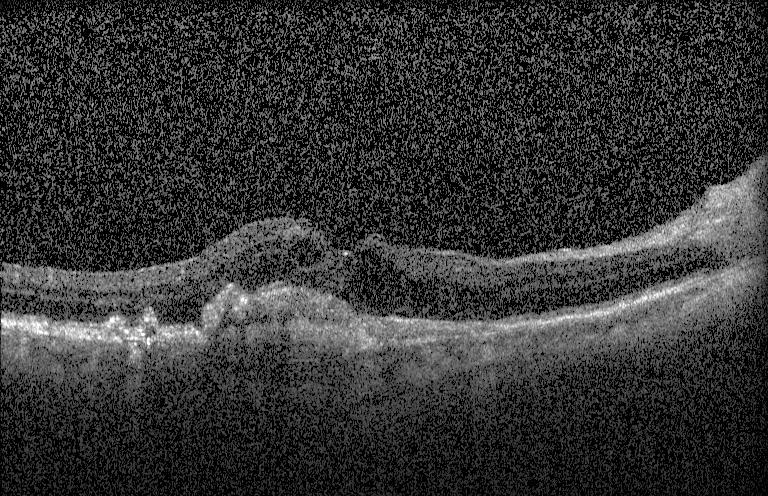
Optical coherence tomography scan, centered on the fovea — Finding: choroidal neovascularization (CNV).